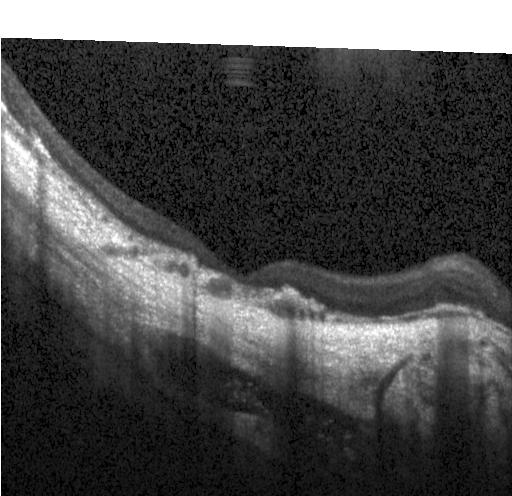
Spectral-domain optical coherence tomography, acquired on a Heidelberg Spectralis, fovea-centered, optical coherence tomography B-scan. Dx: choroidal neovascularization.